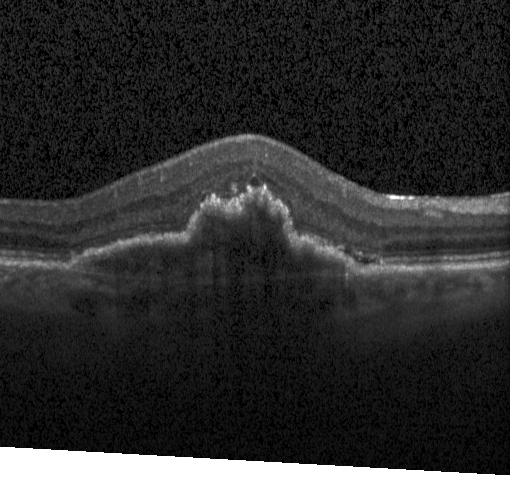 Optical coherence tomography scan.
Impression: CNV.